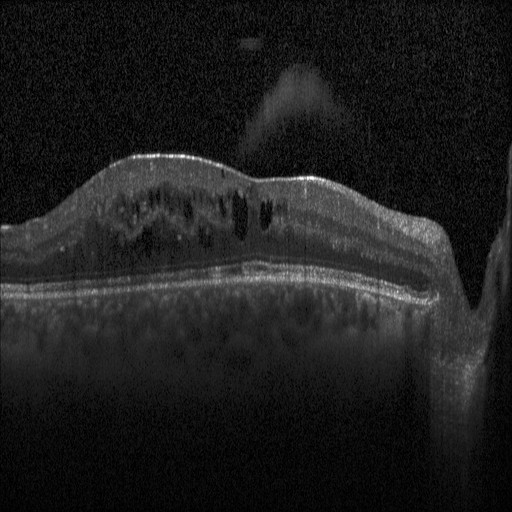
Centered on the fovea. Retinal OCT B-scan. Finding: diabetic macular edema (DME).